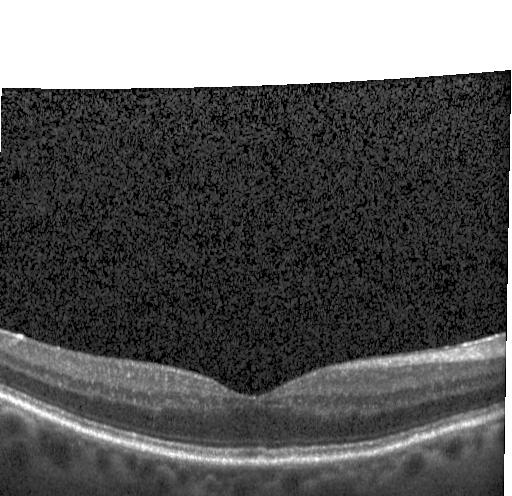 Optical coherence tomography scan · horizontal scan through the fovea · Heidelberg Spectralis. Dx: neither CNV, DME, nor drusen.